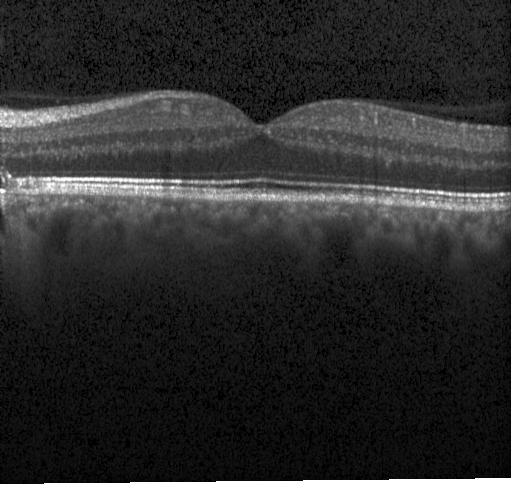
This B-scan demonstrates neither choroidal neovascularization, diabetic macular edema, nor drusen.